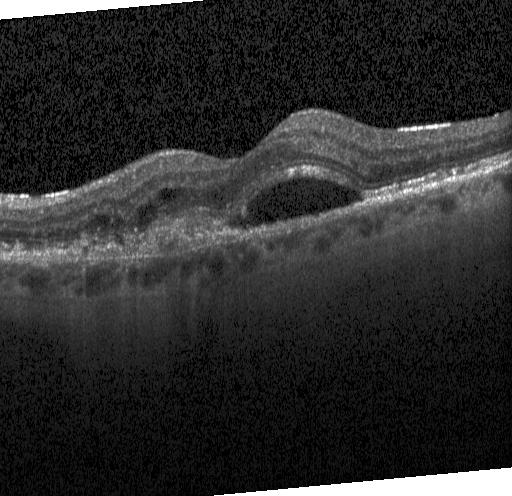
OCT line scan. Heidelberg Spectralis. Centered on the fovea
Diagnosis: CNV.